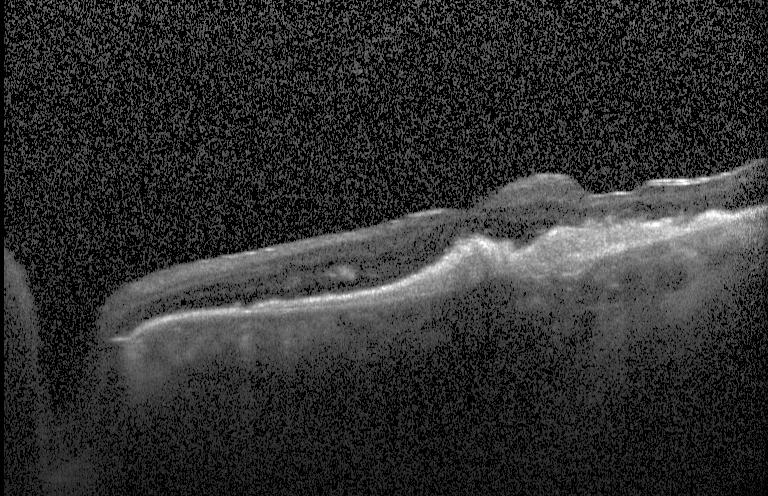

Dx: a choroidal neovascular membrane.